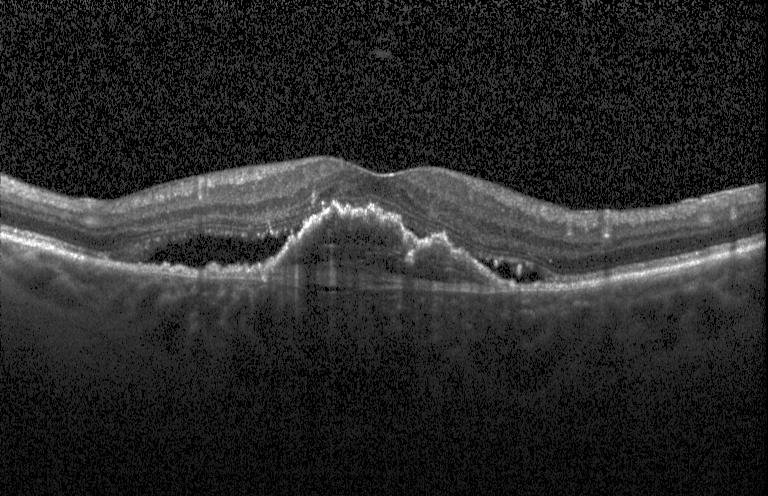
Fovea-centered · OCT line scan · instrument: Heidelberg Spectralis.
OCT finding: a choroidal neovascular membrane.